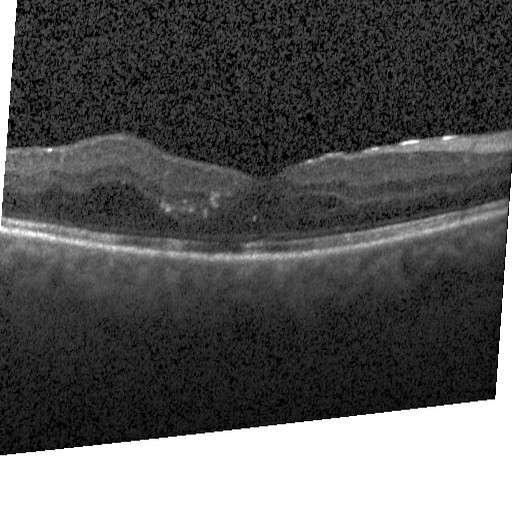

Spectral-domain OCT, Heidelberg Spectralis, optical coherence tomography B-scan.
Assessment: DME.